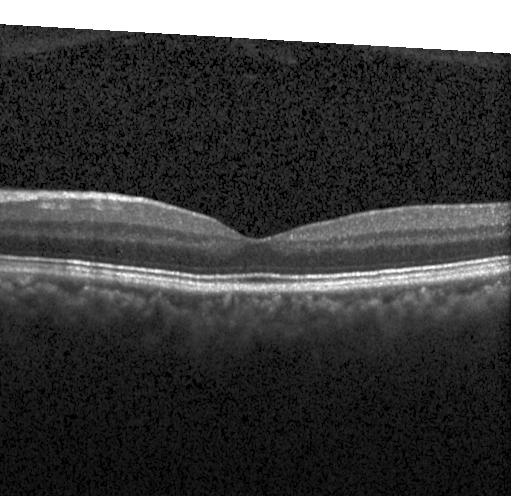 Instrument: Heidelberg Spectralis; through the macula; spectral-domain OCT; OCT line scan.
Macular OCT: no CNV, DME, or drusen.